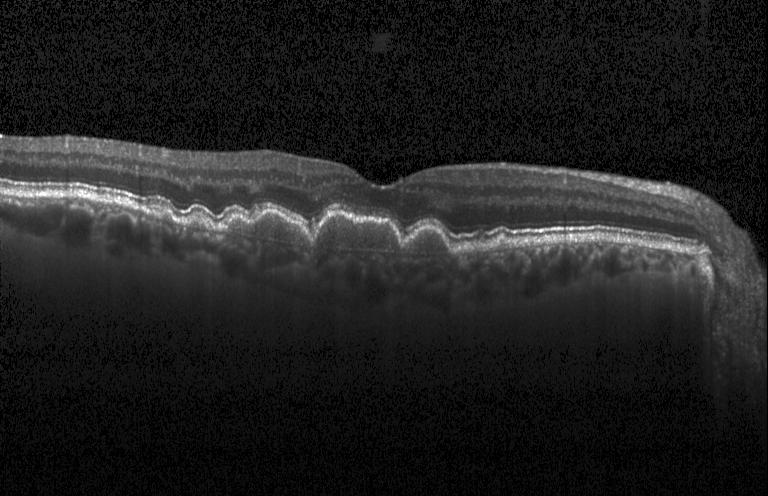 Acquired on a Heidelberg Spectralis · OCT line scan · through the macula · spectral-domain OCT
OCT finding: multiple drusen.